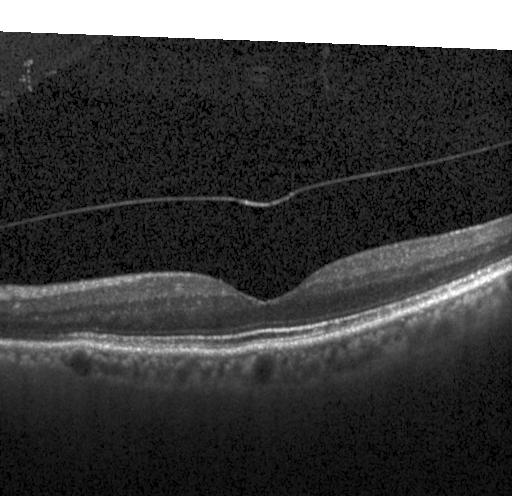 OCT line scan.
Diagnosis: no CNV, no DME, and no drusen.